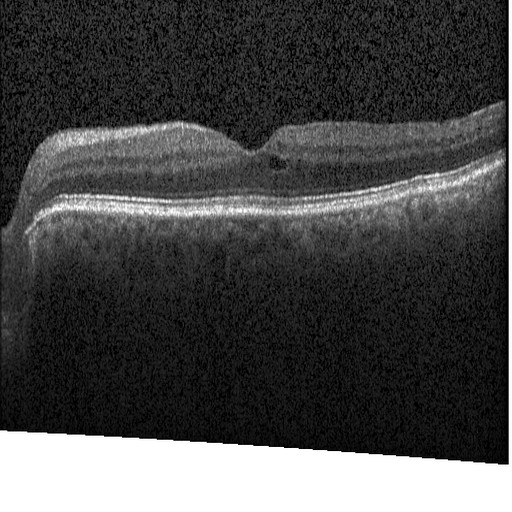
Horizontal scan through the fovea · retinal OCT cross-section. This B-scan demonstrates diabetic macular edema.